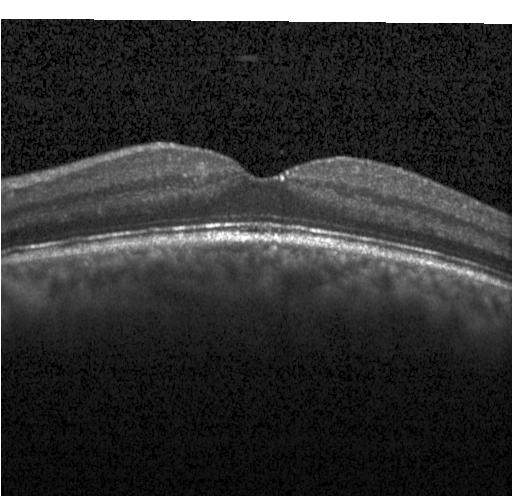

OCT line scan, macular scan.
Neither CNV, DME, nor drusen.